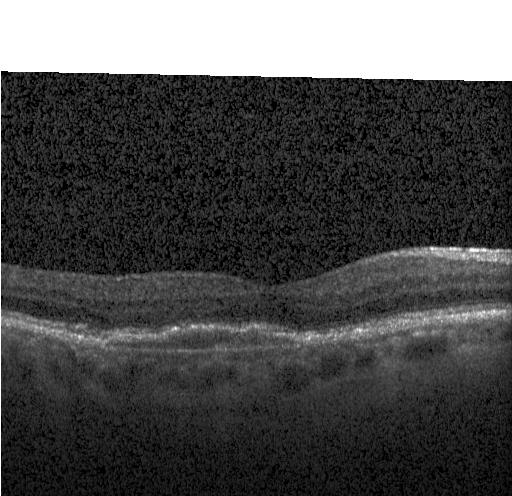 Through the macula · optical coherence tomography scan · SD-OCT. This B-scan demonstrates CNV.